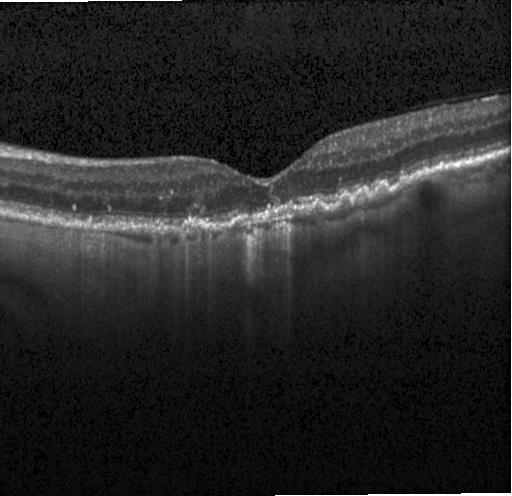 Impression: sub-RPE drusenoid deposits.